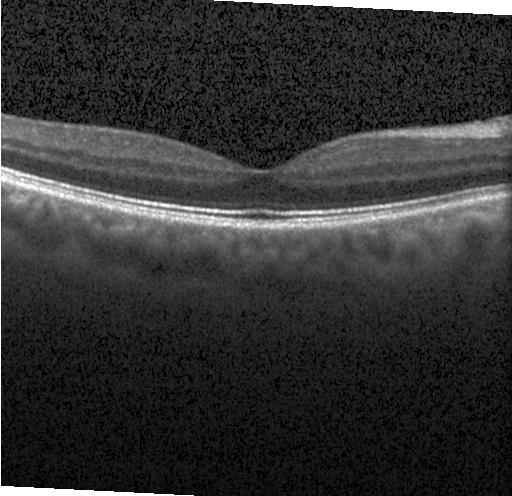

Heidelberg Spectralis. Macular scan. Retinal OCT B-scan. Impression: no evidence of choroidal neovascularization, diabetic macular edema, or drusen.